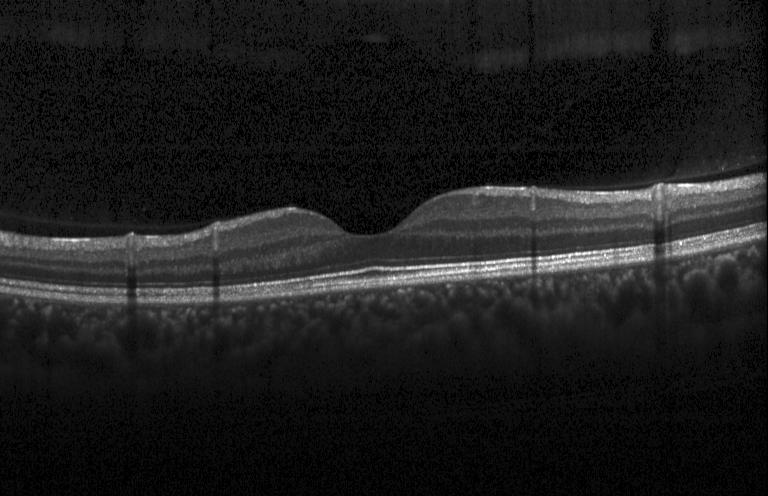

Through the macula, acquired on a Heidelberg Spectralis, OCT line scan — This B-scan demonstrates no CNV, DME, or drusen.